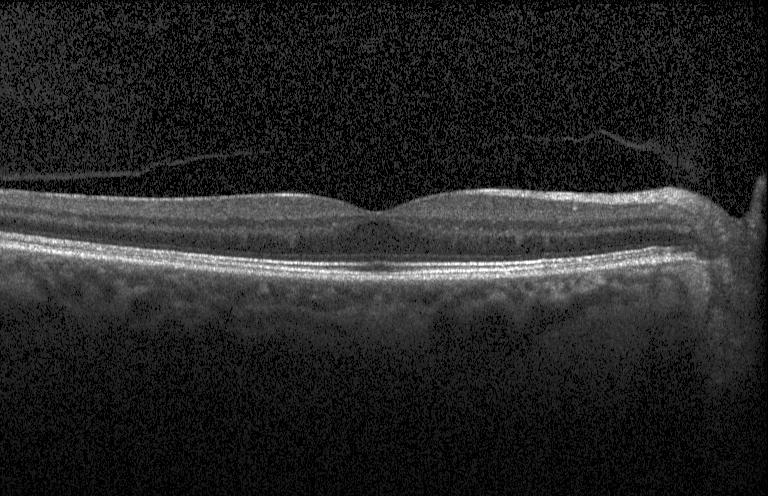

Spectral-domain OCT B-scan: neither CNV, DME, nor drusen.